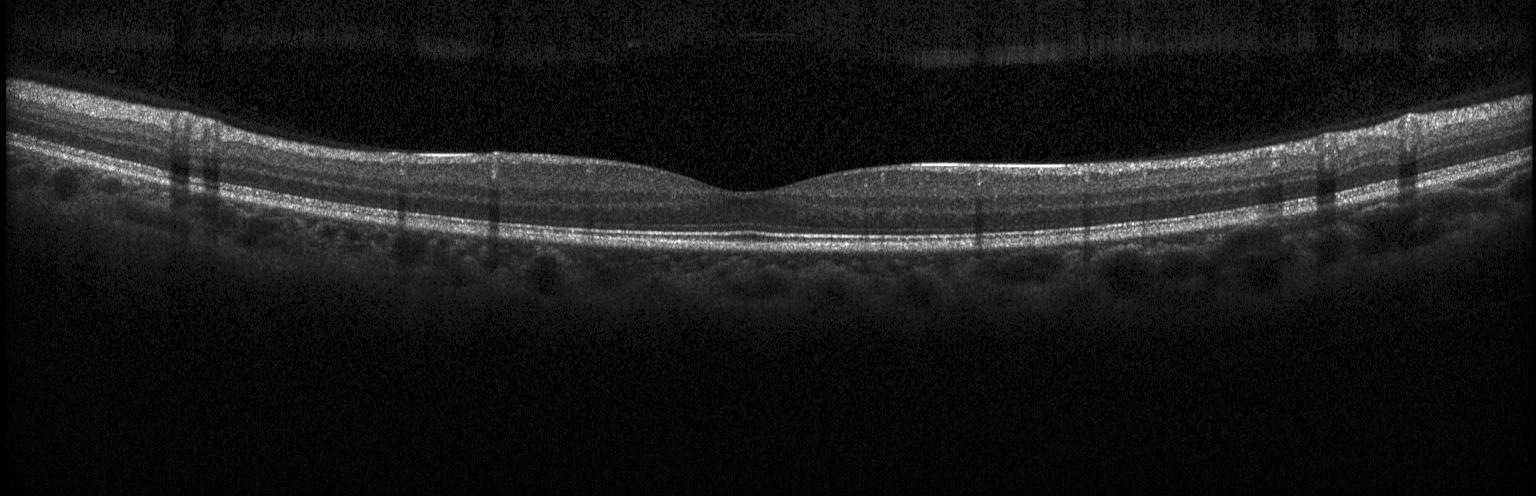
This B-scan demonstrates no evidence of choroidal neovascularization, diabetic macular edema, or drusen.